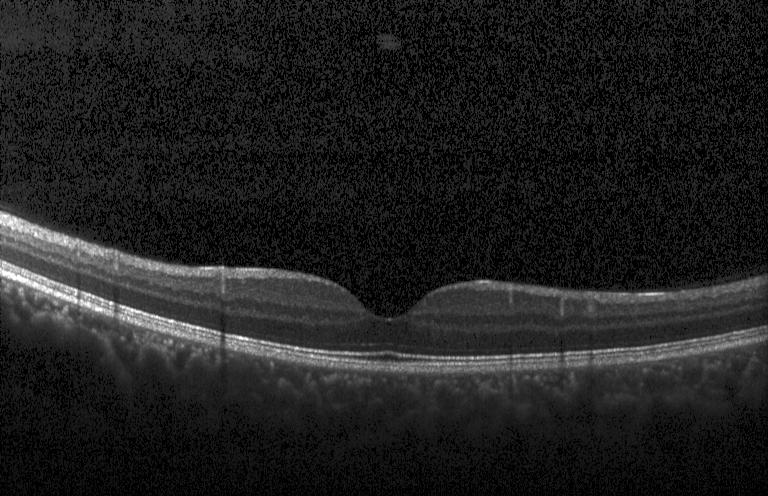

Macular OCT: no choroidal neovascularization, diabetic macular edema, or drusen.